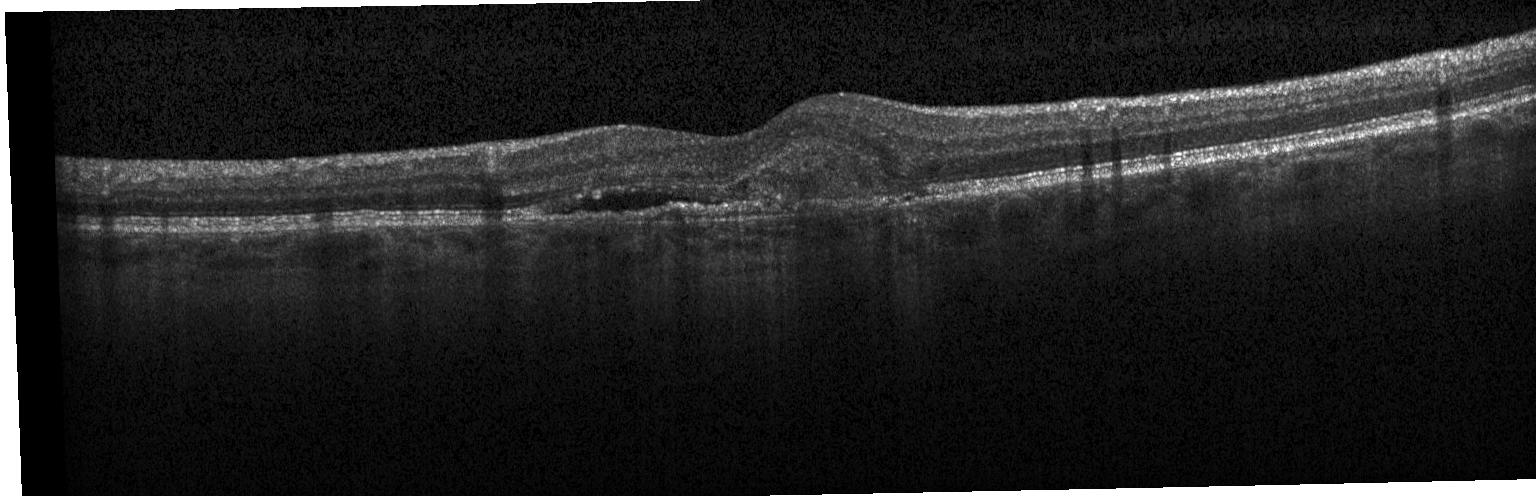

OCT line scan. Diagnosis: choroidal neovascularization.